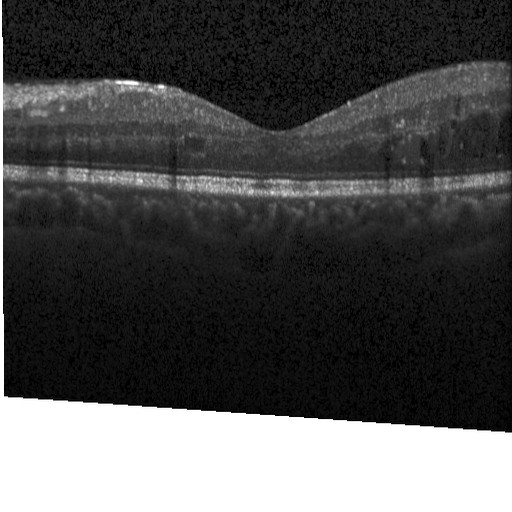 Diagnosis: DME.